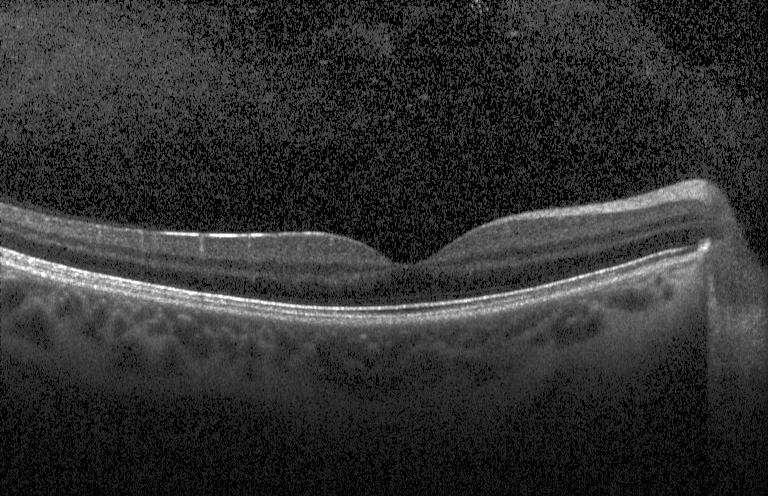

Assessment: no evidence of choroidal neovascularization, diabetic macular edema, or drusen.